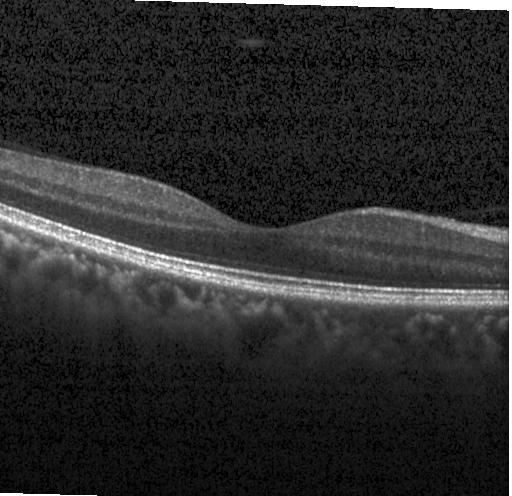
OCT finding: no evidence of CNV, DME, or drusen.